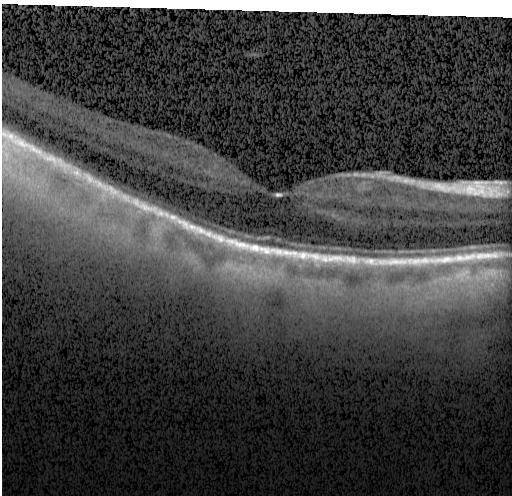 Macular OCT demonstrating no choroidal neovascularization, no diabetic macular edema, and no drusen.